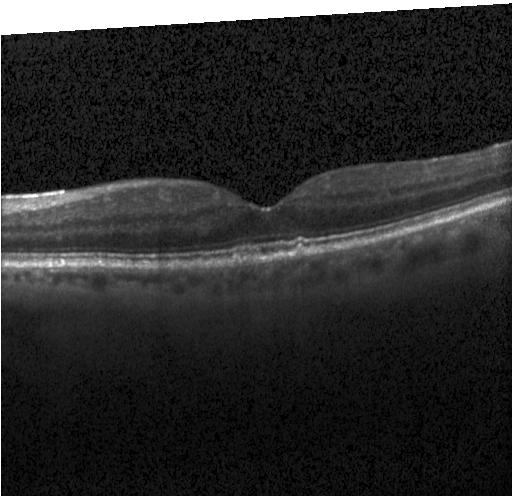 Heidelberg Spectralis OCT system. OCT B-scan. Spectral-domain optical coherence tomography.
Finding: multiple drusen.